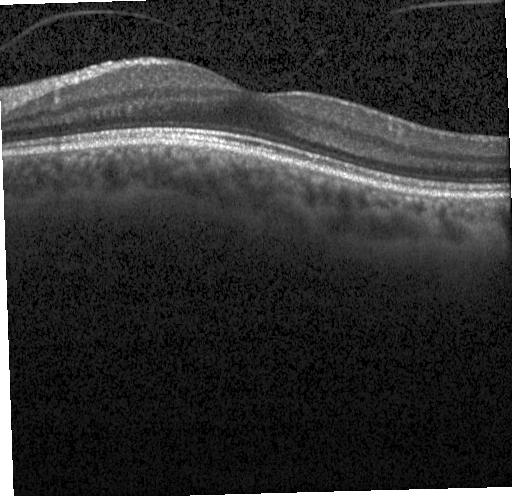 Finding: no choroidal neovascularization, diabetic macular edema, or drusen.